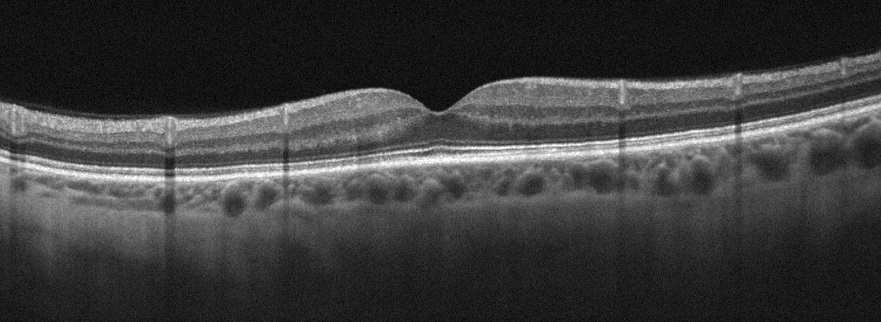

The scan shows no AMD, DME, ERM, RAO, RVO, or VID.